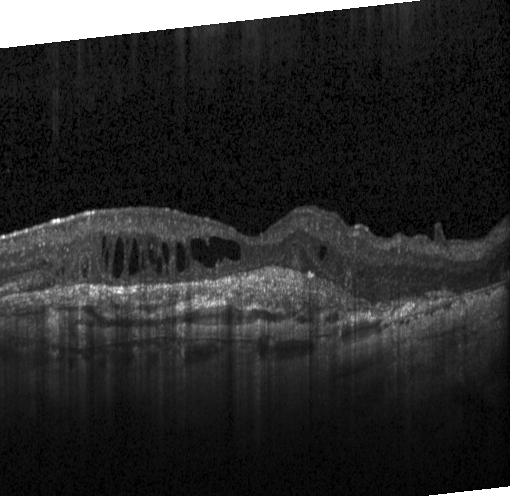 Assessment: a choroidal neovascular membrane.